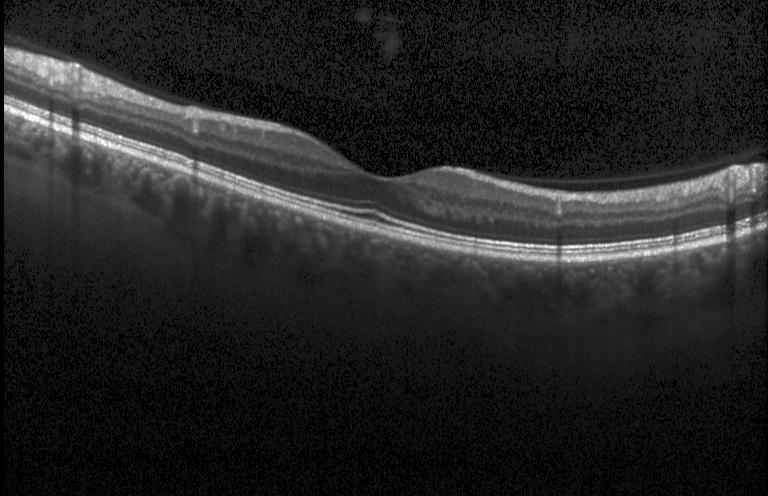

OCT line scan; SD-OCT; acquired on a Heidelberg Spectralis.
The scan shows no CNV, no DME, and no drusen.